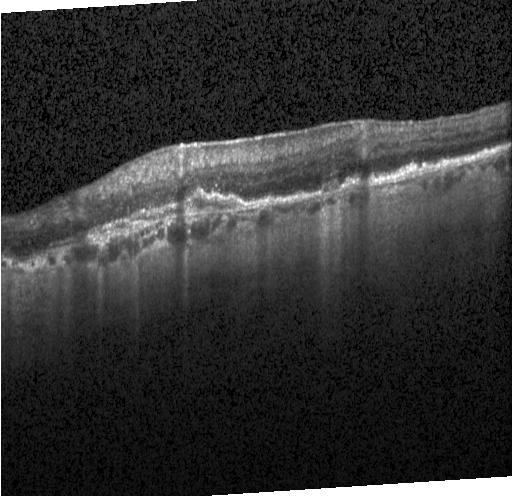 Optical coherence tomography scan, Heidelberg Spectralis OCT system, SD-OCT, through the macula.
Assessment: a choroidal neovascular membrane.